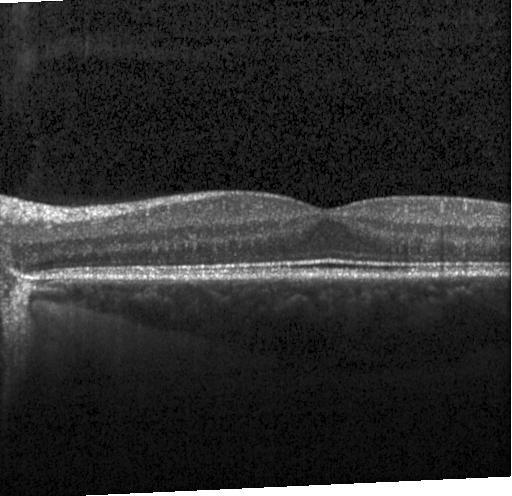
Instrument: Heidelberg Spectralis; optical coherence tomography B-scan
Assessment: no evidence of choroidal neovascularization, diabetic macular edema, or drusen.